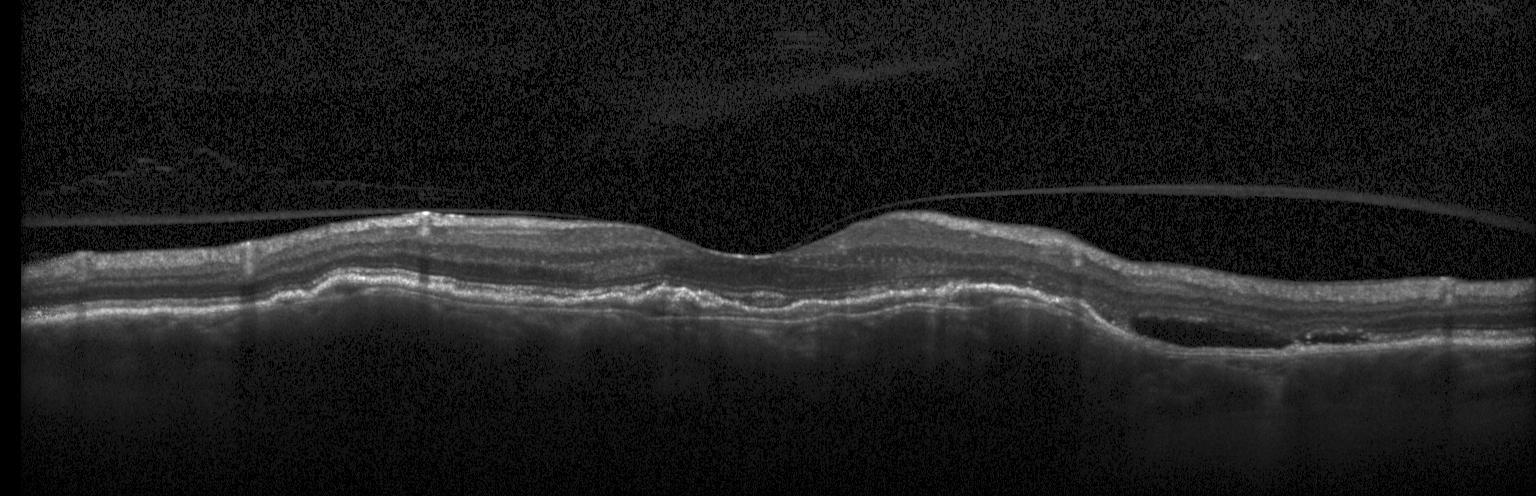
Macular scan; spectral-domain OCT; retinal OCT cross-section
Dx: a choroidal neovascular membrane.